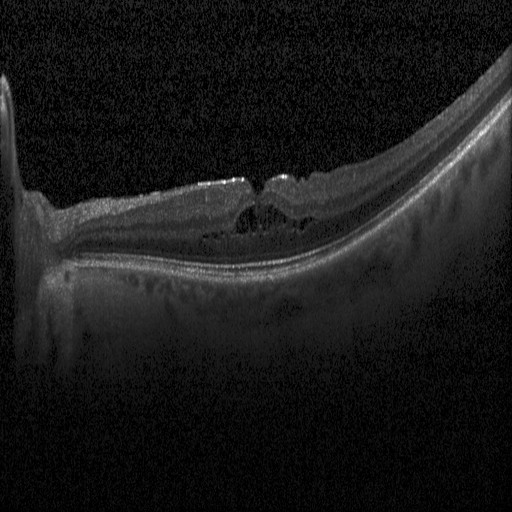
Retinal OCT cross-section showing DME.